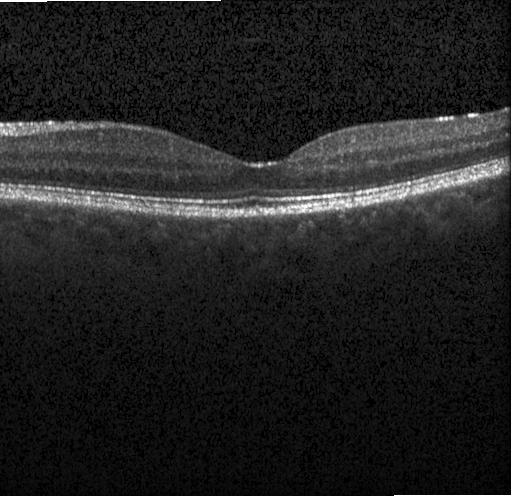
OCT B-scan. The scan shows no CNV, DME, or drusen.